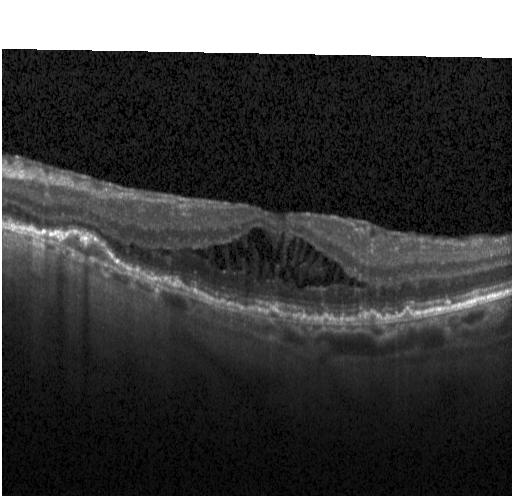
OCT line scan — Finding: DME.